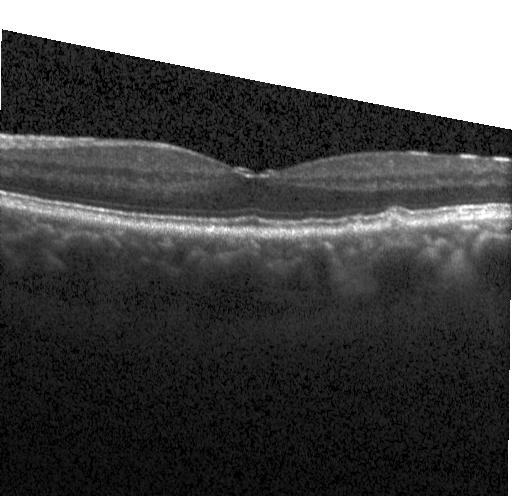 OCT B-scan, centered on the fovea, Heidelberg Spectralis
Diagnosis: multiple drusen.